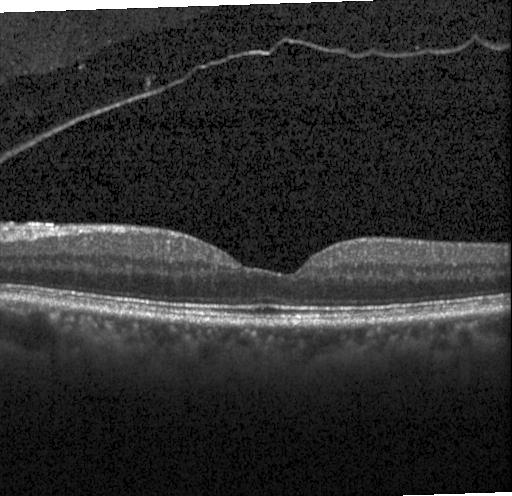
Finding: no evidence of choroidal neovascularization, diabetic macular edema, or drusen.